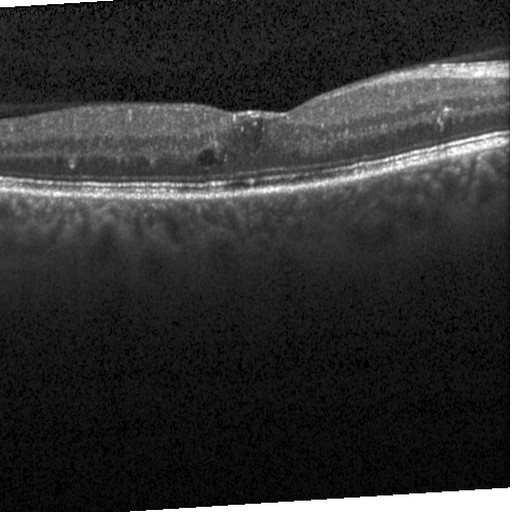

Optical coherence tomography scan · Heidelberg Spectralis OCT system · fovea-centered.
Diagnosis: diabetic macular edema (DME).